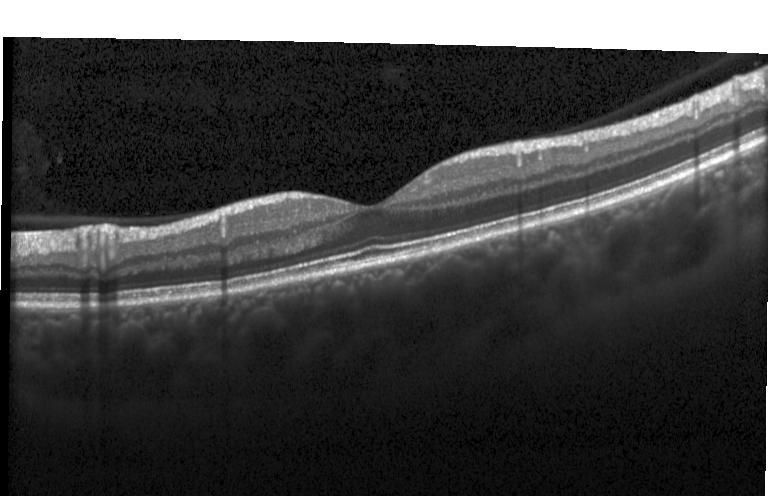 Retinal OCT cross-section showing no CNV, no DME, and no drusen.